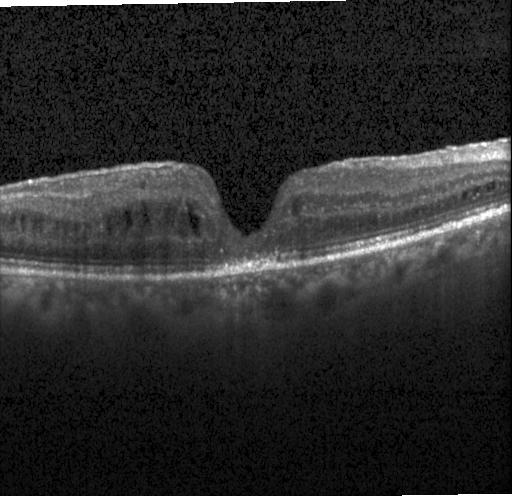 DME.